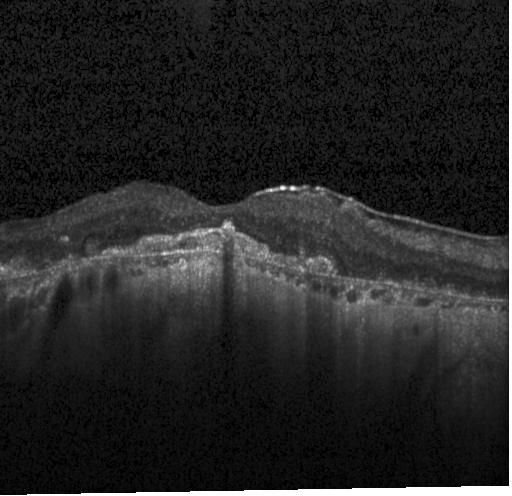
OCT B-scan, through the macula, Heidelberg Spectralis.
The scan shows a choroidal neovascular membrane.